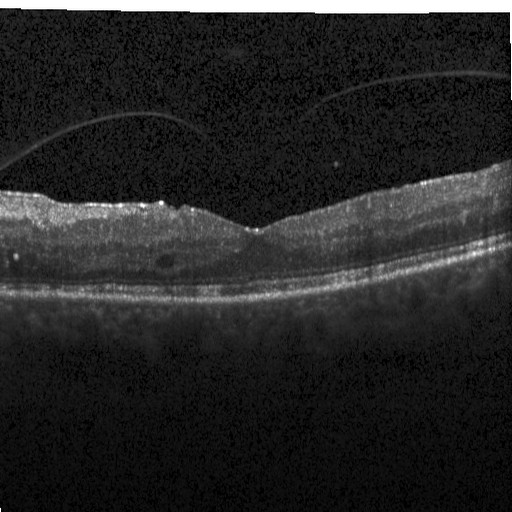 Macular scan. Spectral-domain optical coherence tomography. Heidelberg Spectralis. Retinal OCT B-scan. Diabetic macular edema.